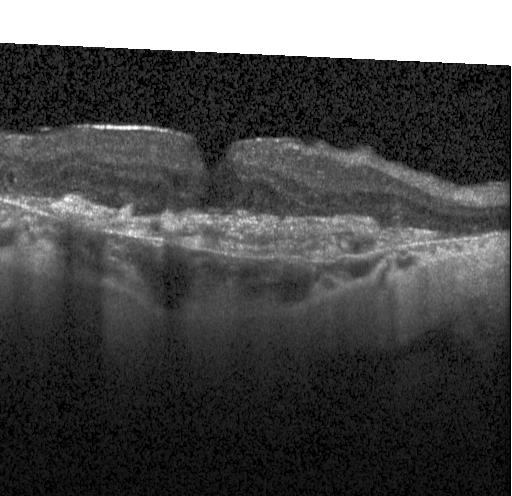
OCT B-scan · Heidelberg Spectralis OCT system · through the macula.
Diagnosis: a choroidal neovascular membrane.